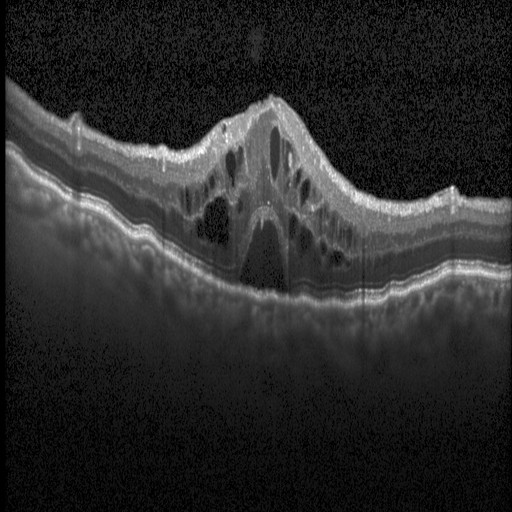

Heidelberg Spectralis OCT system, retinal OCT B-scan, spectral-domain optical coherence tomography, horizontal scan through the fovea — Finding: DME.